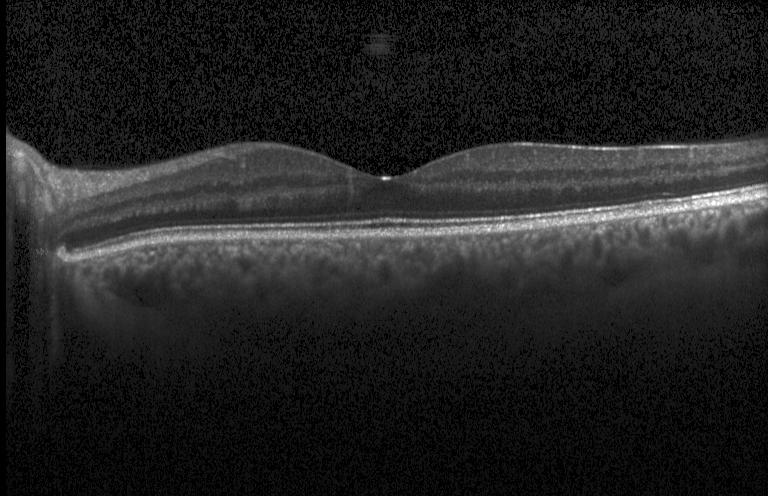
Macular OCT: neither choroidal neovascularization, diabetic macular edema, nor drusen.